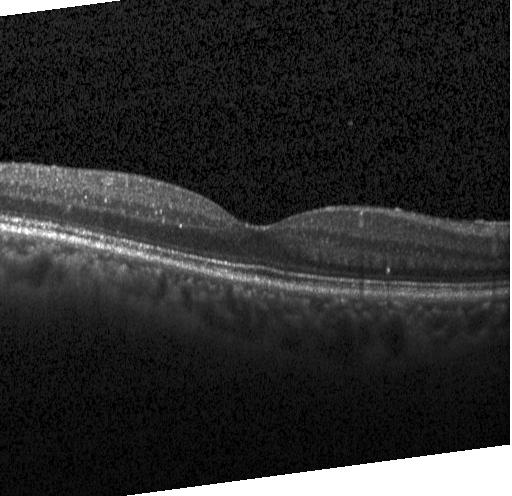 OCT B-scan showing no evidence of choroidal neovascularization, diabetic macular edema, or drusen.